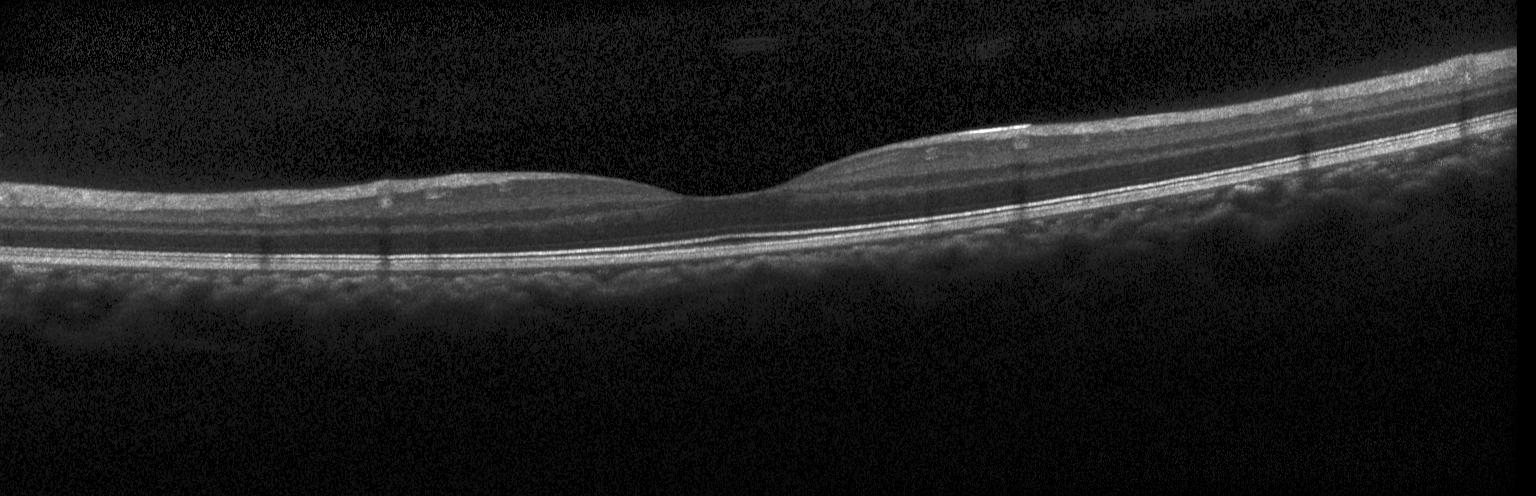

Spectral-domain OCT · OCT B-scan — This B-scan demonstrates no evidence of choroidal neovascularization, diabetic macular edema, or drusen.